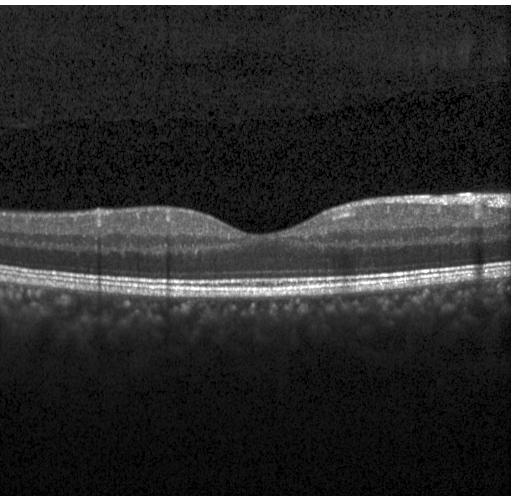

Fovea-centered; acquired on a Heidelberg Spectralis; OCT B-scan. This B-scan demonstrates no choroidal neovascularization, no diabetic macular edema, and no drusen.